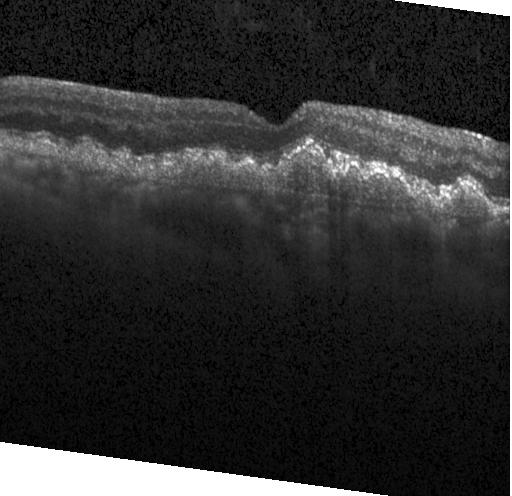
OCT scan showing a choroidal neovascular membrane.